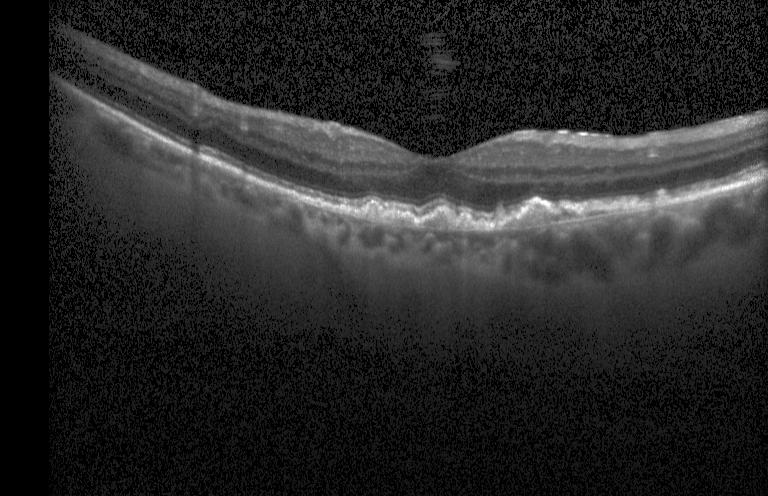

Horizontal scan through the fovea · Heidelberg Spectralis · SD-OCT · retinal OCT B-scan.
Diagnosis: sub-RPE drusenoid deposits.